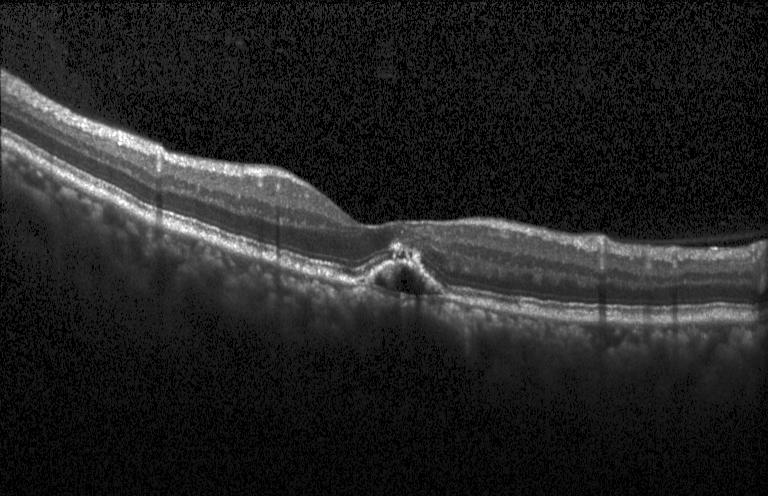
A choroidal neovascular membrane.